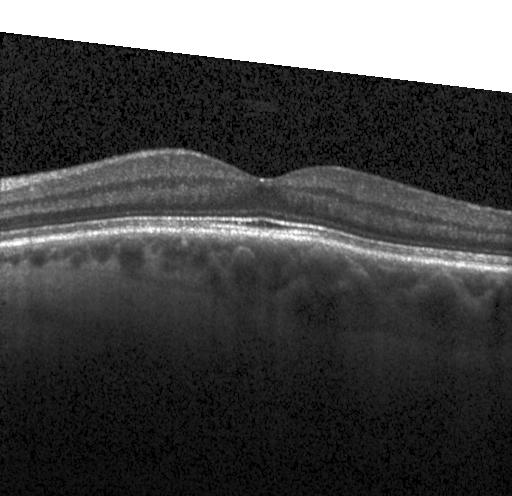
Optical coherence tomography scan
Assessment: no choroidal neovascularization, diabetic macular edema, or drusen.